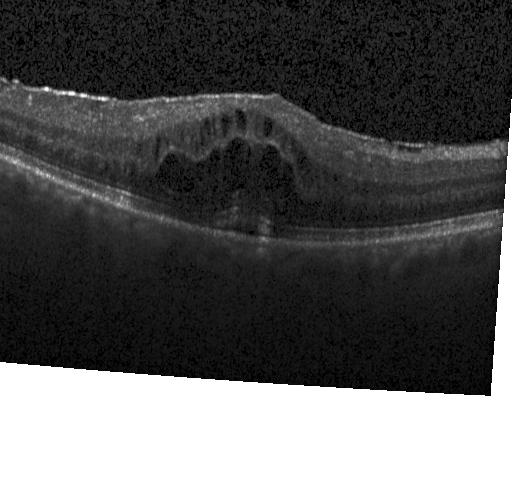 Spectral-domain OCT. Optical coherence tomography scan. Macular OCT: diabetic macular edema.